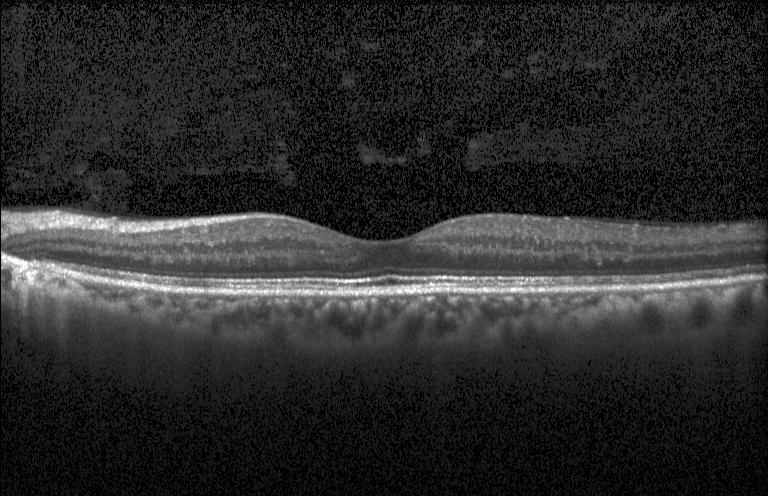
Retinal OCT B-scan · instrument: Heidelberg Spectralis — No evidence of choroidal neovascularization, diabetic macular edema, or drusen.